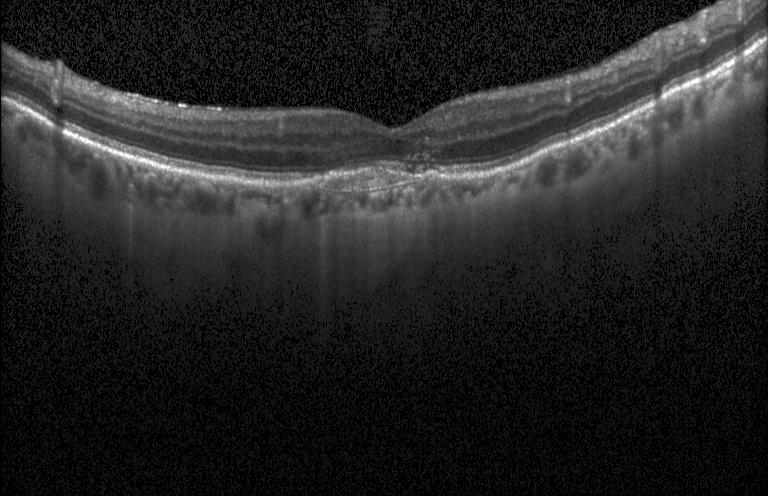
OCT line scan · instrument: Heidelberg Spectralis · through the macula · spectral-domain OCT
Diagnosis: choroidal neovascularization (CNV).